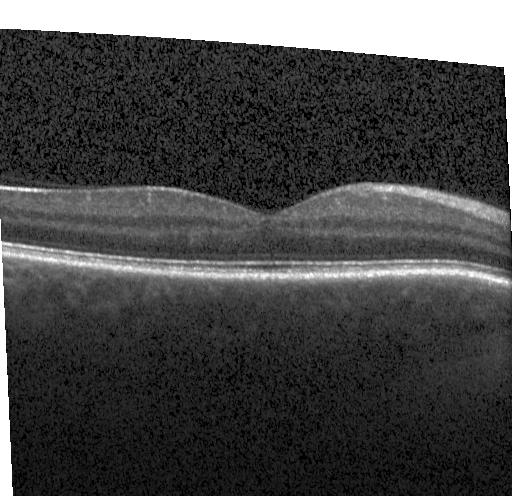
Spectral-domain OCT B-scan: no choroidal neovascularization, diabetic macular edema, or drusen.